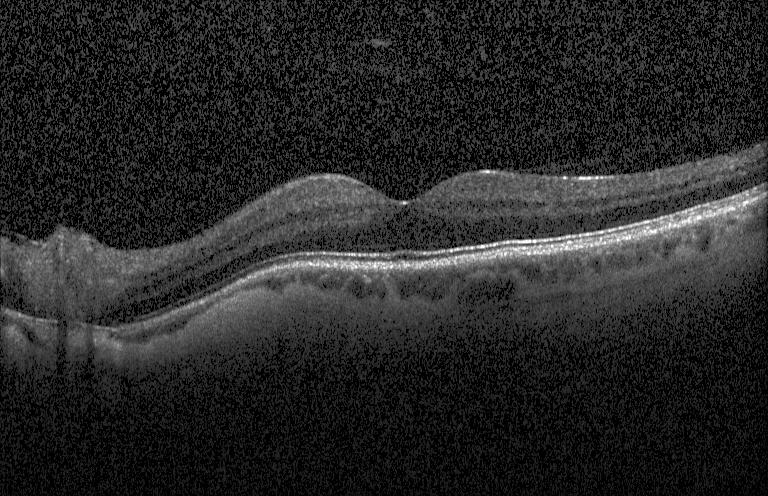 Optical coherence tomography B-scan. Fovea-centered.
No evidence of choroidal neovascularization, diabetic macular edema, or drusen.